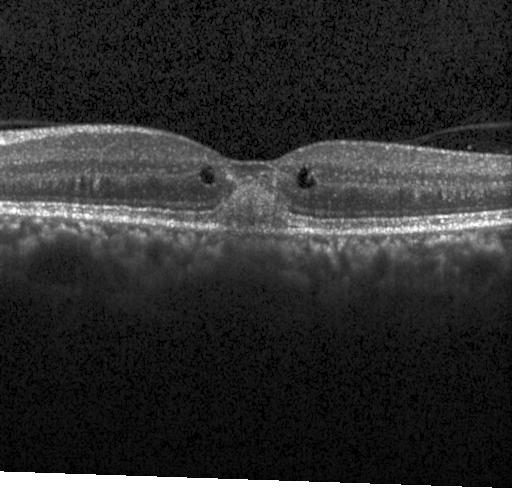 Finding: a choroidal neovascular membrane.